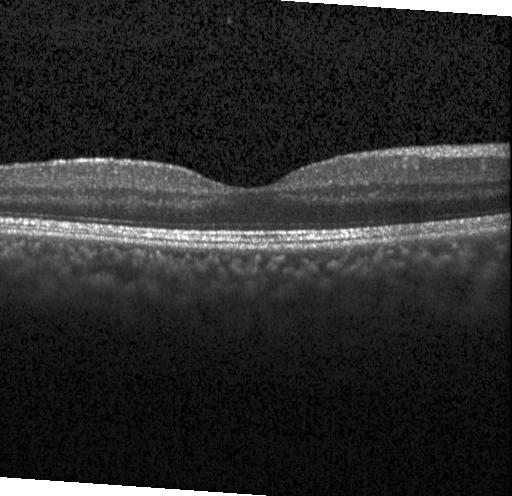

Macular scan · acquired on a Heidelberg Spectralis · OCT line scan.
Diagnosis: neither CNV, DME, nor drusen.